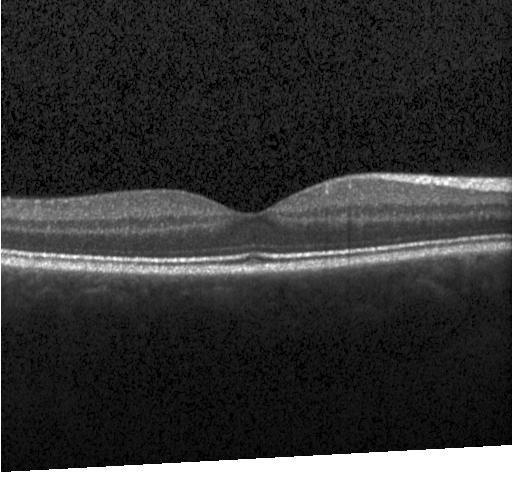 Retinal OCT cross-section.
Assessment: no choroidal neovascularization, no diabetic macular edema, and no drusen.